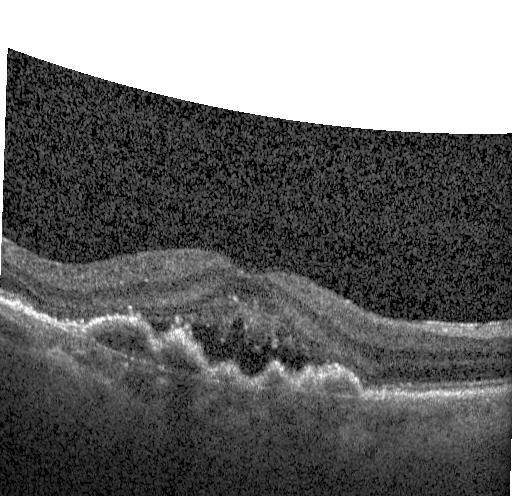 Spectral-domain OCT B-scan: a choroidal neovascular membrane.